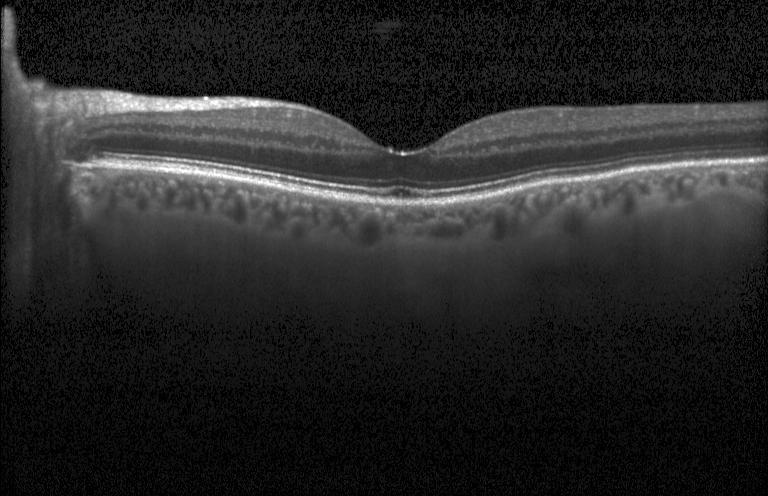
Heidelberg Spectralis OCT system. OCT B-scan. Diagnosis: no evidence of choroidal neovascularization, diabetic macular edema, or drusen.